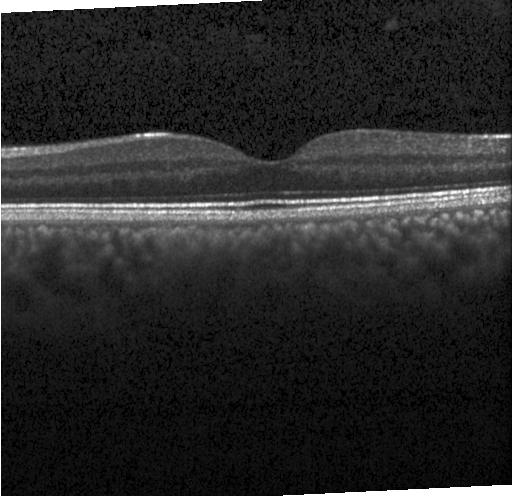

Spectral-domain OCT B-scan: neither CNV, DME, nor drusen.